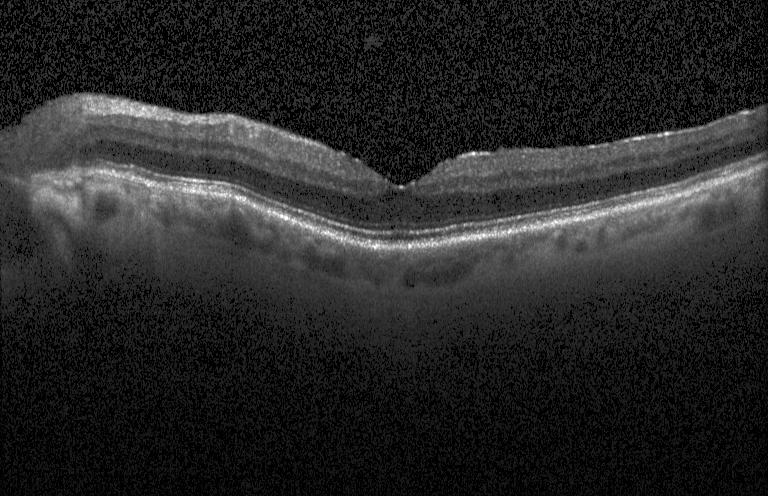

Retinal OCT cross-section. SD-OCT. Through the macula — Macular OCT: neither CNV, DME, nor drusen.